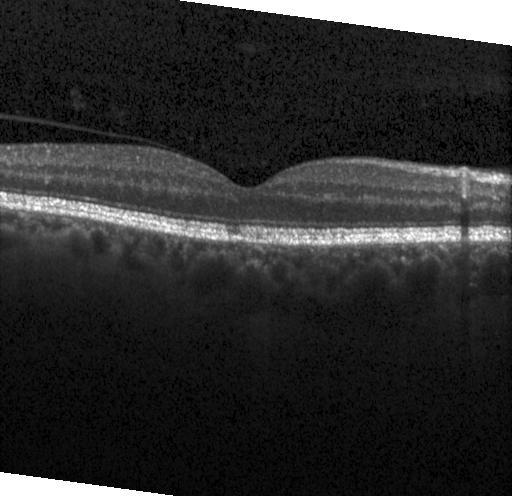 SD-OCT, OCT B-scan.
Impression: no CNV, DME, or drusen.